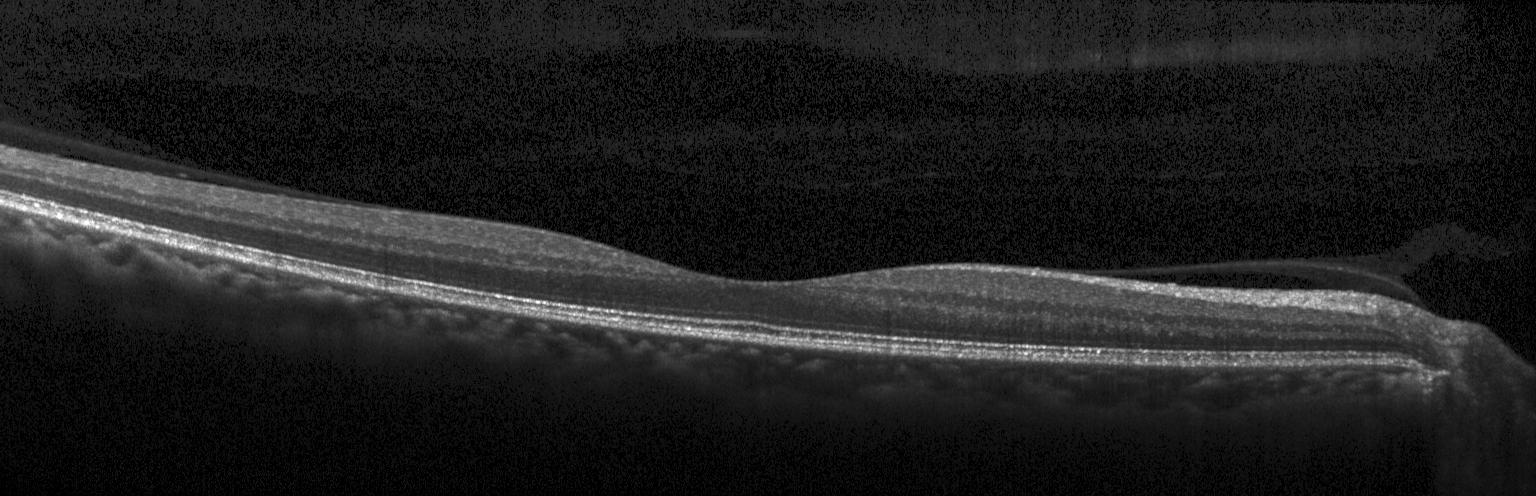 Horizontal scan through the fovea; acquired on a Heidelberg Spectralis; spectral-domain OCT; optical coherence tomography B-scan — Impression: no CNV, no DME, and no drusen.